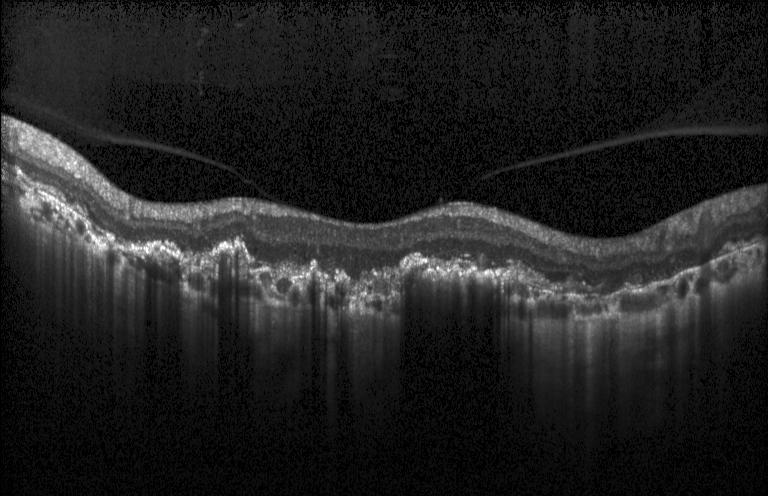 Retinal OCT B-scan · spectral-domain OCT — Macular OCT: a choroidal neovascular membrane.